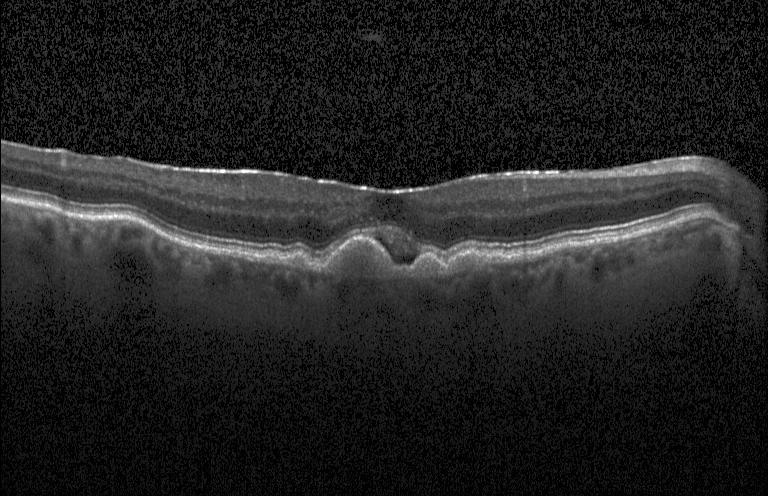

OCT B-scan
This B-scan demonstrates multiple drusen.